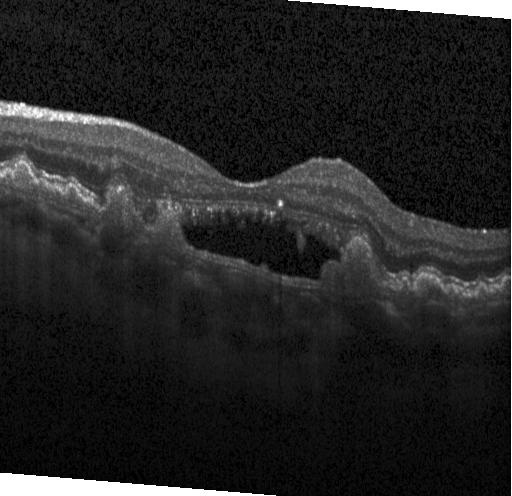
OCT B-scan showing CNV.